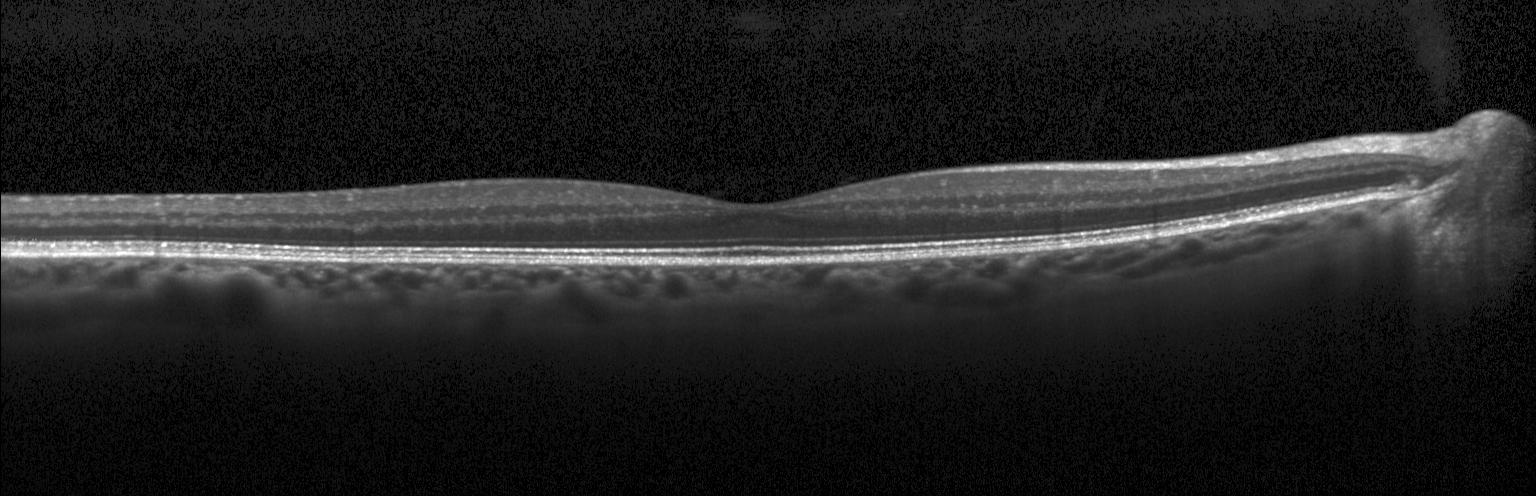 Optical coherence tomography scan, centered on the fovea, Heidelberg Spectralis OCT system, spectral-domain optical coherence tomography — No choroidal neovascularization, no diabetic macular edema, and no drusen.